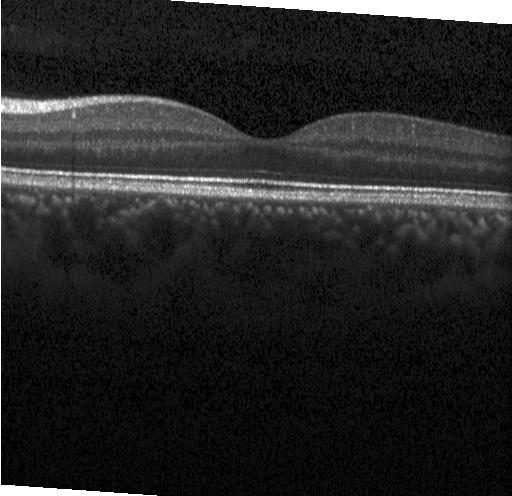

Macular OCT demonstrating neither choroidal neovascularization, diabetic macular edema, nor drusen.